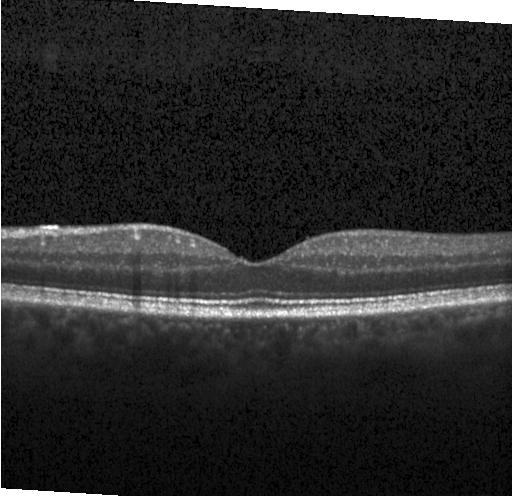
Retinal OCT cross-section showing neither choroidal neovascularization, diabetic macular edema, nor drusen.